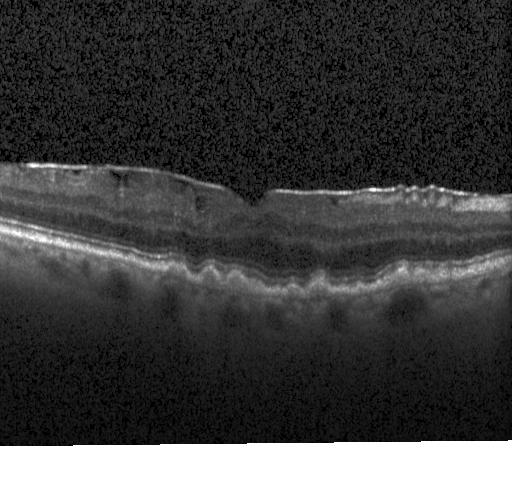
Spectral-domain OCT B-scan: sub-RPE drusenoid deposits.